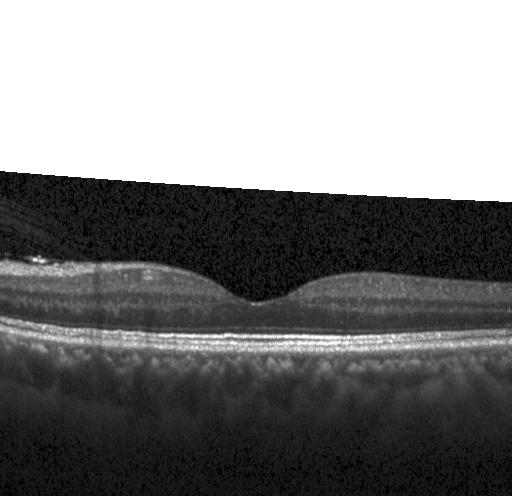
Retinal OCT cross-section; centered on the fovea; instrument: Heidelberg Spectralis. Impression: neither choroidal neovascularization, diabetic macular edema, nor drusen.